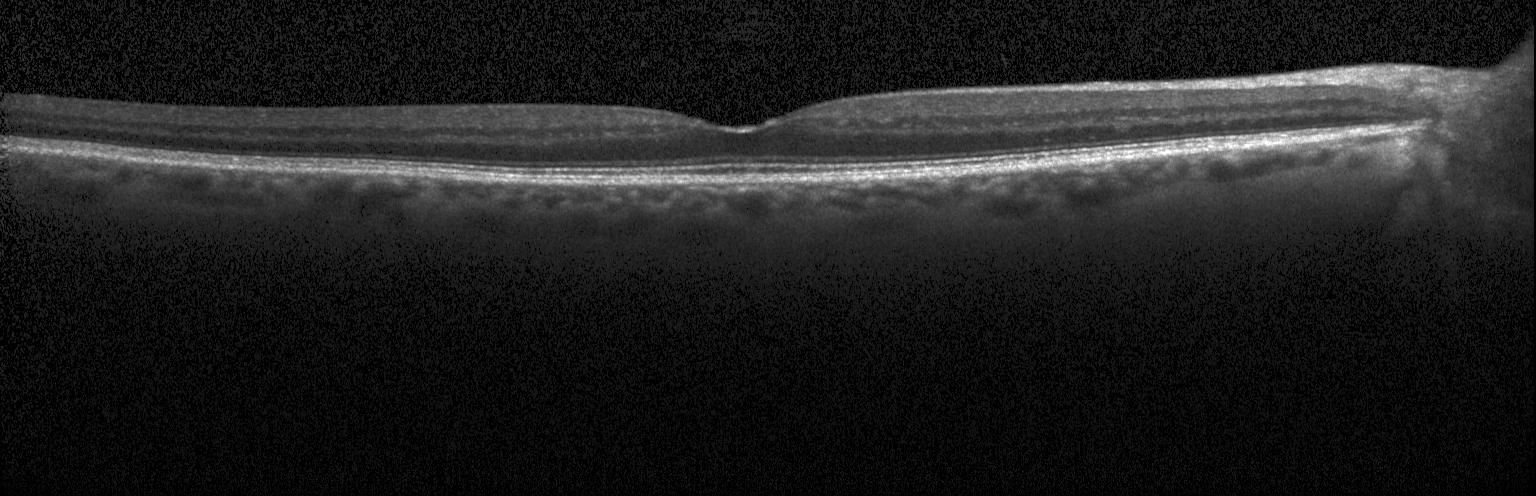

Retinal OCT cross-section
Macular OCT: no evidence of choroidal neovascularization, diabetic macular edema, or drusen.